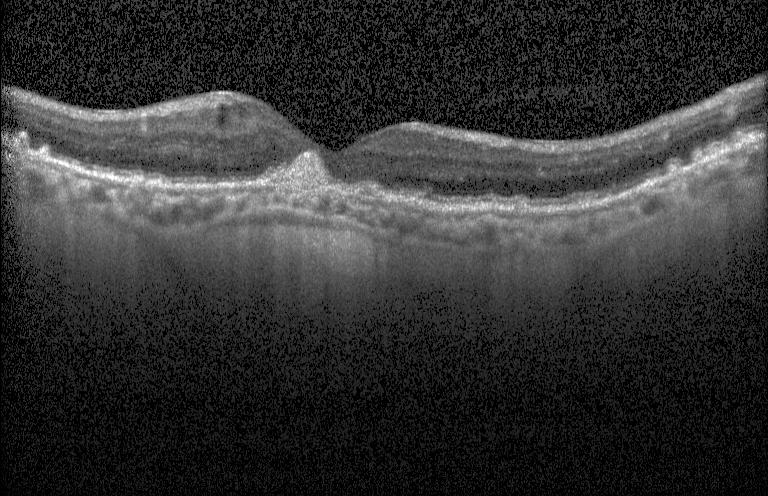

Dx: a choroidal neovascular membrane.